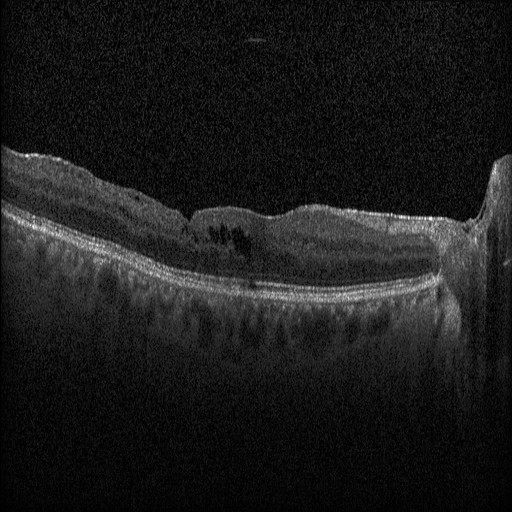 The scan shows DME.